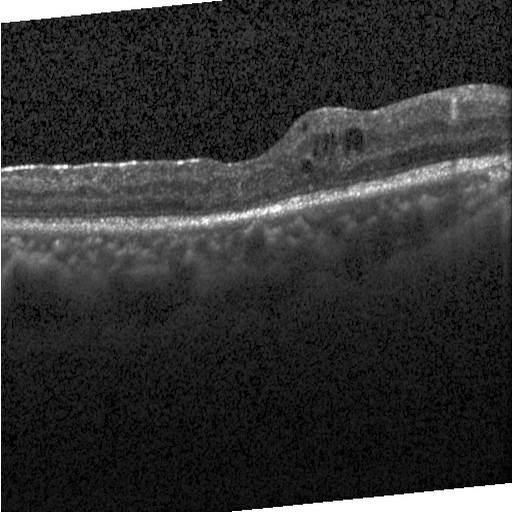
Acquired on a Heidelberg Spectralis, retinal OCT B-scan, centered on the fovea, SD-OCT. Diabetic macular edema (DME).